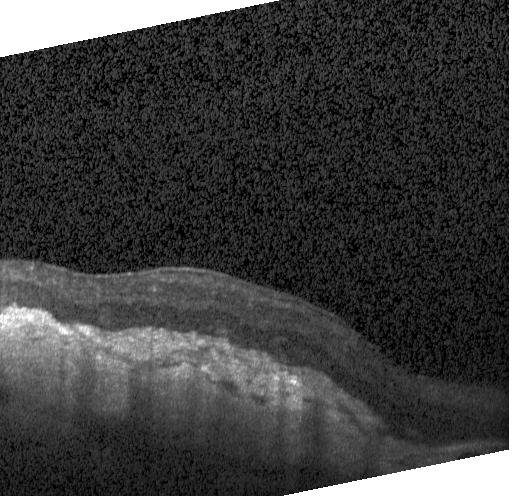

Fovea-centered · retinal OCT B-scan · spectral-domain OCT. The scan shows choroidal neovascularization.